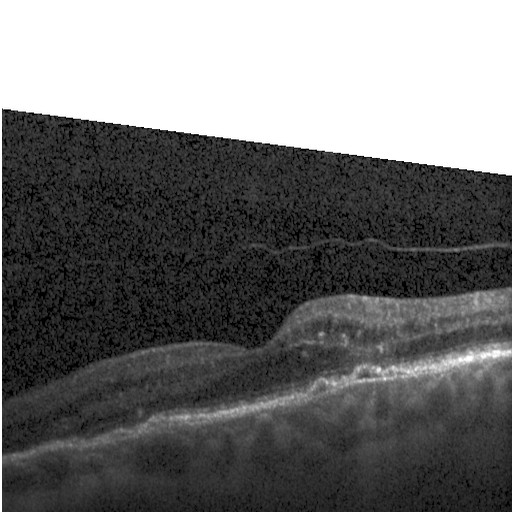
Spectral-domain OCT. Heidelberg Spectralis OCT system. Retinal OCT cross-section. Through the macula.
Impression: DME.